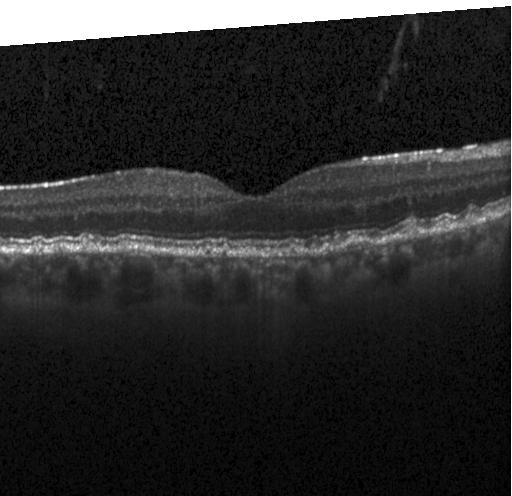 Macular scan · Heidelberg Spectralis · spectral-domain optical coherence tomography · OCT B-scan. Drusen.